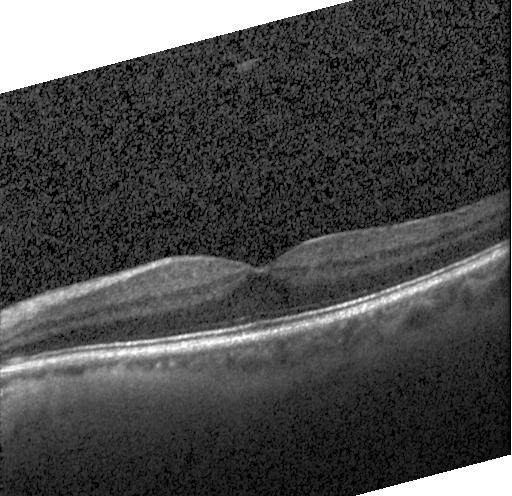
No choroidal neovascularization, diabetic macular edema, or drusen.